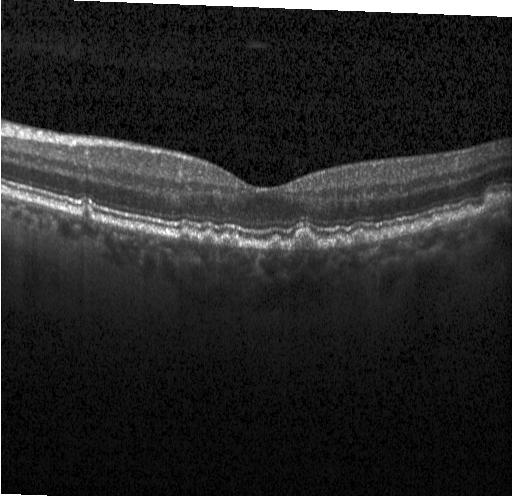

Macular scan; OCT B-scan; spectral-domain OCT; instrument: Heidelberg Spectralis. Finding: drusen.